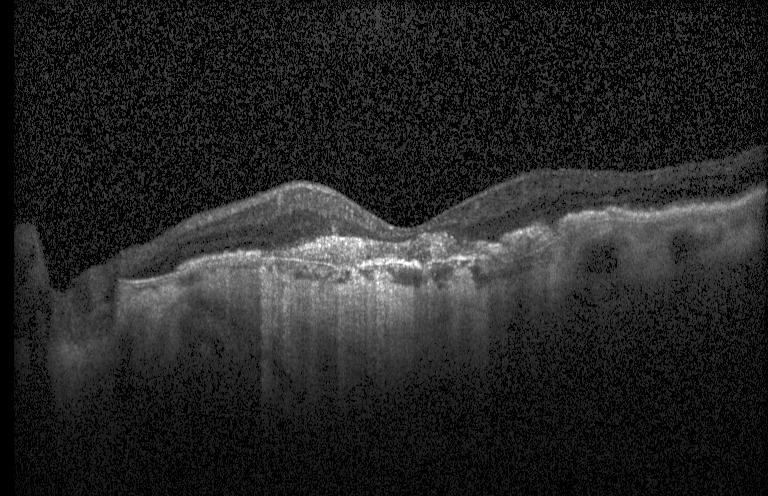

Impression: a choroidal neovascular membrane.